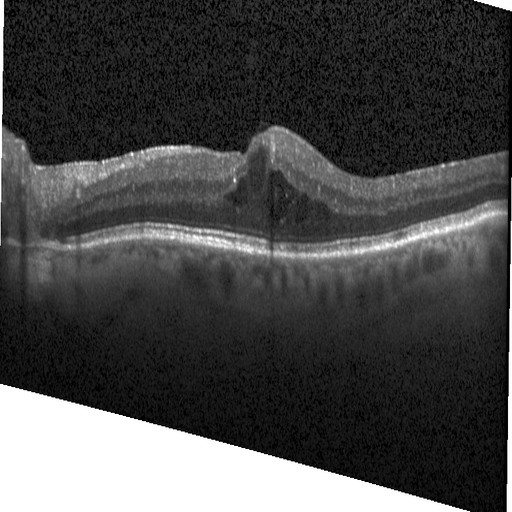
Horizontal scan through the fovea. Retinal OCT cross-section. Acquired on a Heidelberg Spectralis — DME.